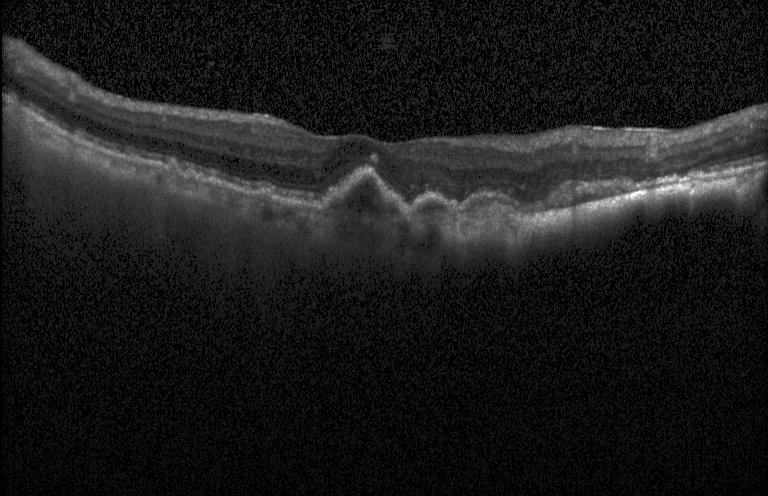

Heidelberg Spectralis. Retinal OCT B-scan. Spectral-domain OCT.
Macular OCT: a choroidal neovascular membrane.